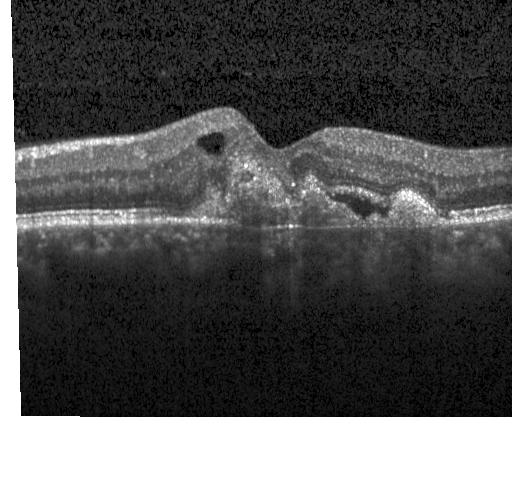
Retinal OCT cross-section
Impression: a choroidal neovascular membrane.